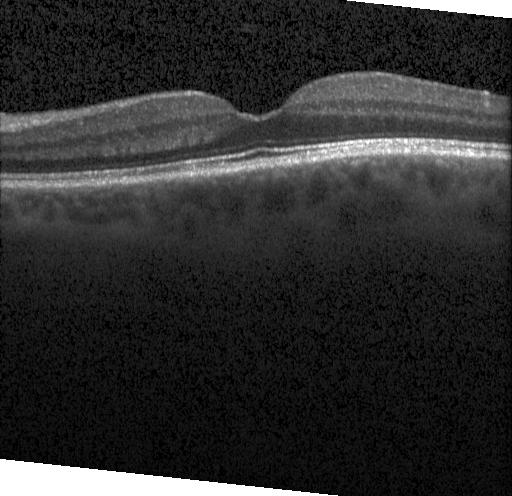

Finding: neither choroidal neovascularization, diabetic macular edema, nor drusen.